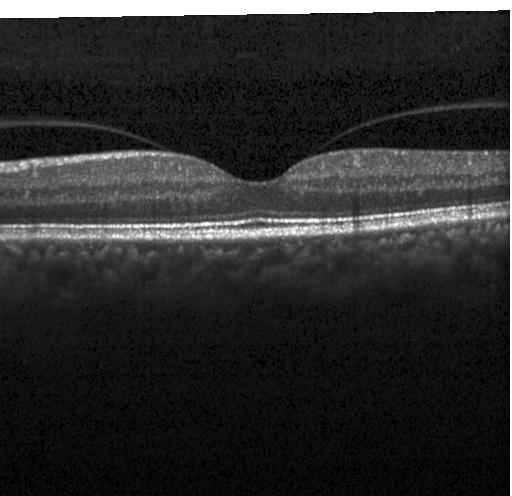

OCT scan showing no choroidal neovascularization, no diabetic macular edema, and no drusen.